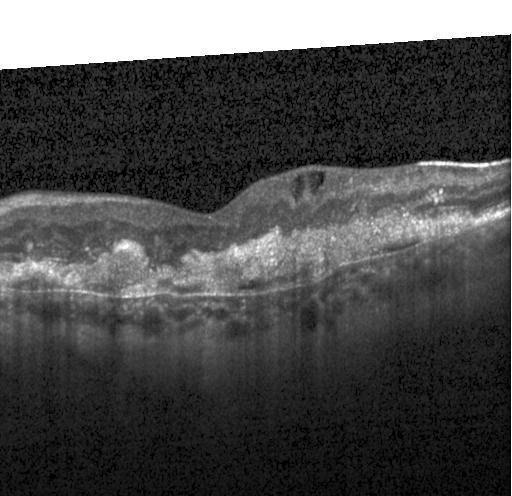
Spectral-domain OCT B-scan: a choroidal neovascular membrane.